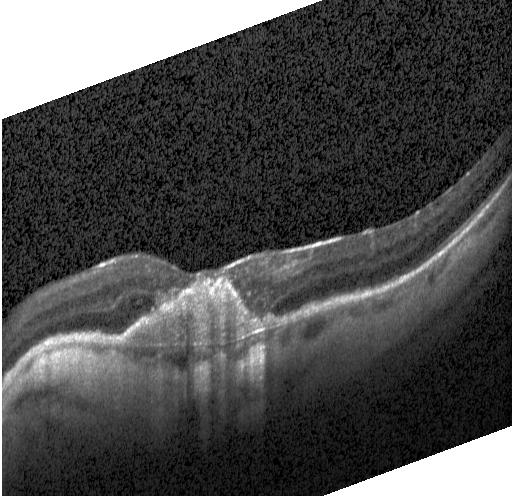

Finding: choroidal neovascularization.